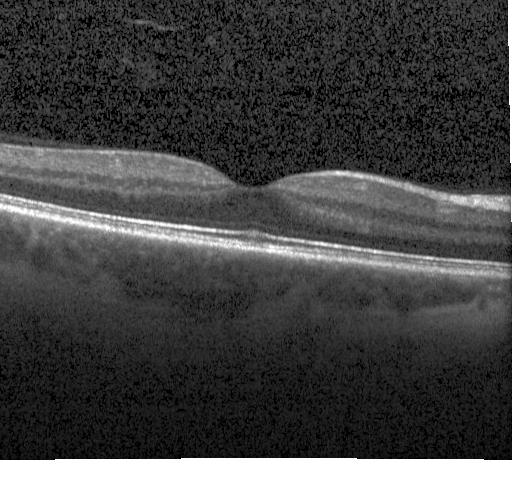

Macular scan; retinal OCT cross-section; spectral-domain optical coherence tomography — Dx: no choroidal neovascularization, no diabetic macular edema, and no drusen.